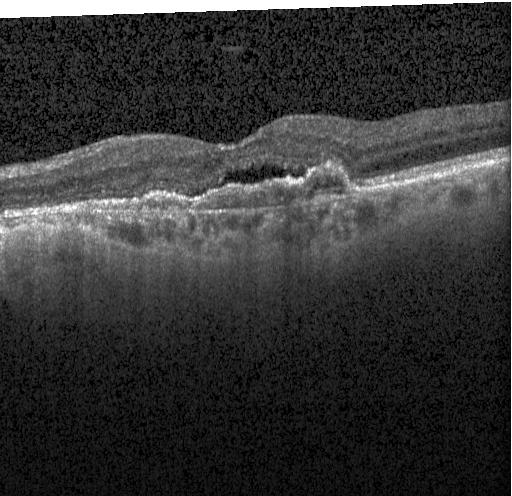

Optical coherence tomography scan · Heidelberg Spectralis OCT system · spectral-domain optical coherence tomography · horizontal scan through the fovea
Diagnosis: CNV.